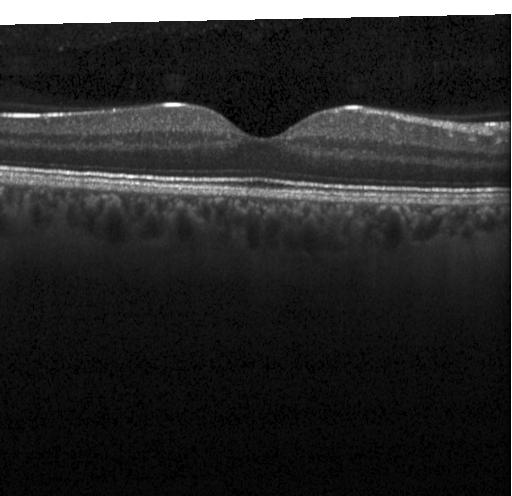
Retinal OCT B-scan; Heidelberg Spectralis OCT system.
Assessment: no evidence of choroidal neovascularization, diabetic macular edema, or drusen.